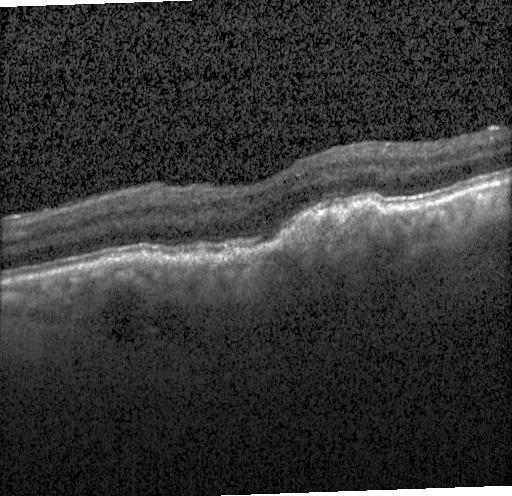 Finding: multiple drusen.